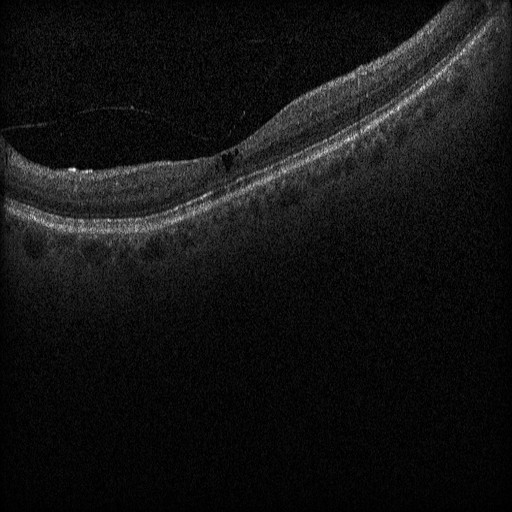
Macular OCT: DME.